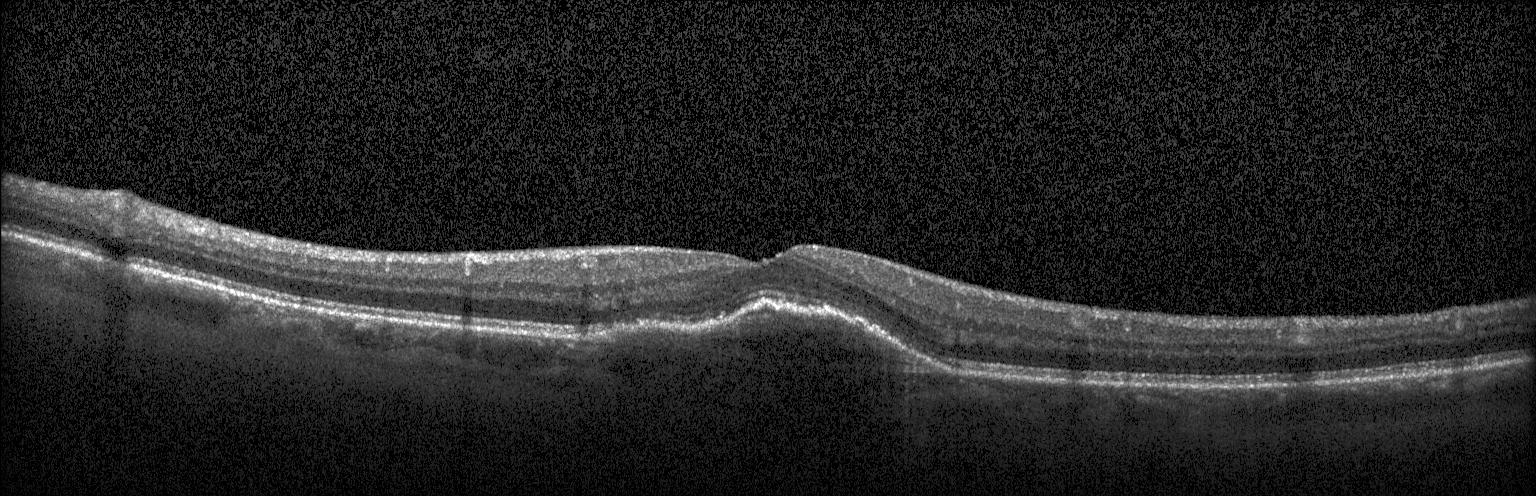
OCT B-scan; through the macula; Heidelberg Spectralis OCT system — Dx: a choroidal neovascular membrane.